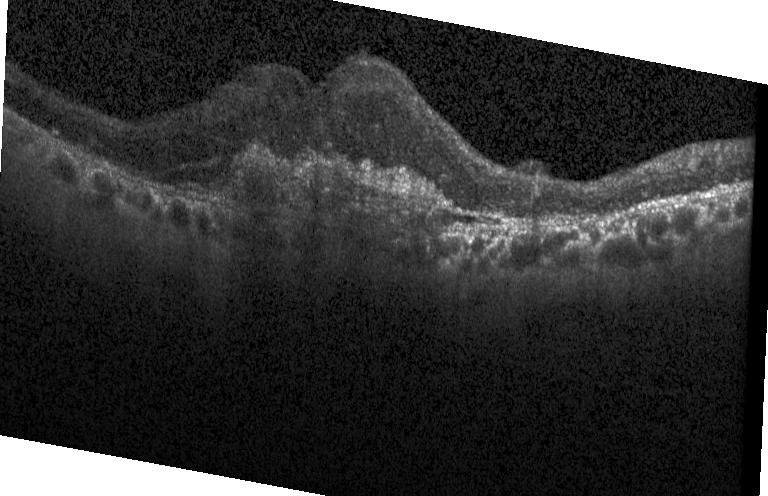
A choroidal neovascular membrane.